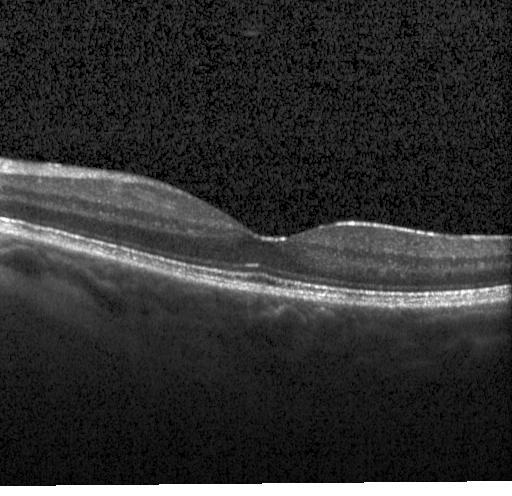 Impression: no CNV, DME, or drusen.